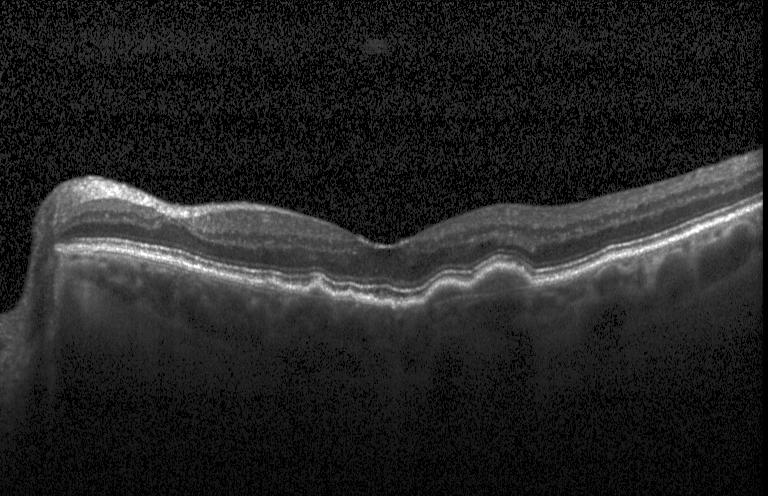

Optical coherence tomography B-scan
Finding: a choroidal neovascular membrane.